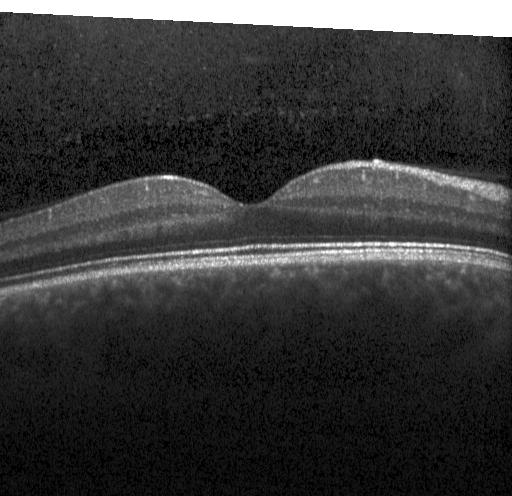

Spectral-domain OCT, Heidelberg Spectralis OCT system, OCT line scan — Diagnosis: no evidence of choroidal neovascularization, diabetic macular edema, or drusen.